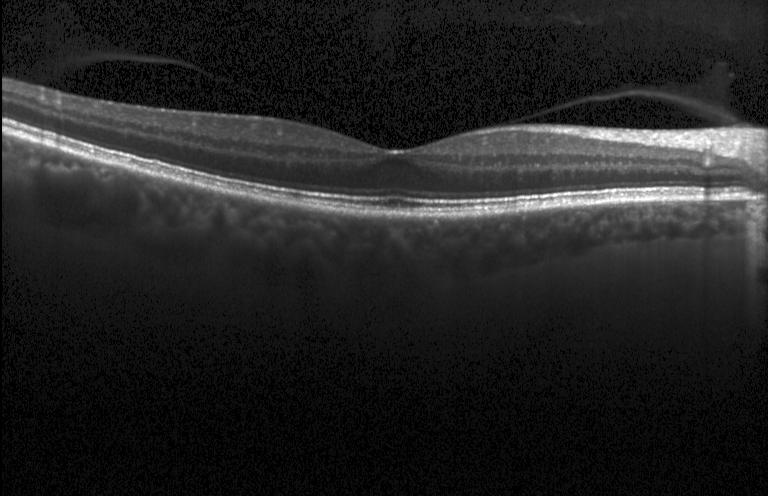 Spectral-domain OCT; retinal OCT B-scan; fovea-centered; Heidelberg Spectralis
Assessment: neither choroidal neovascularization, diabetic macular edema, nor drusen.